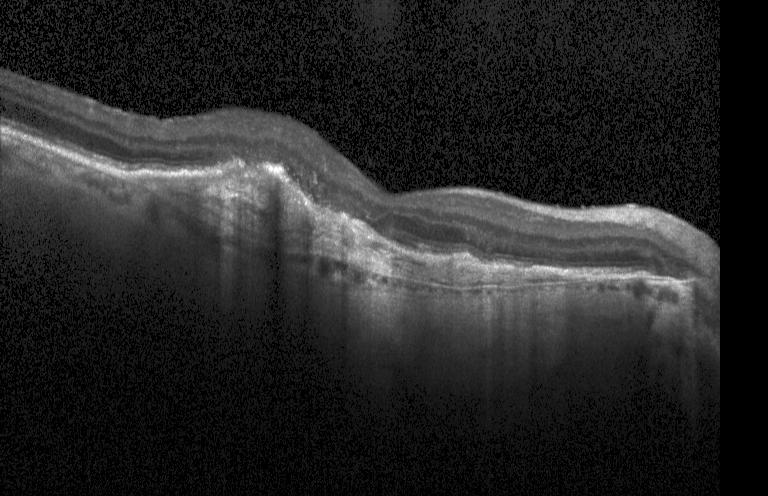

The scan shows a choroidal neovascular membrane.